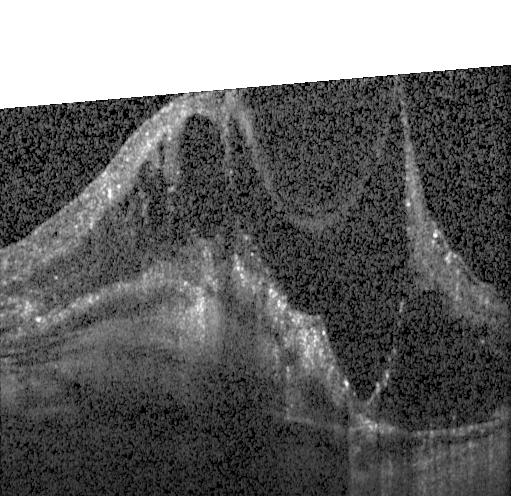

Diagnosis: a choroidal neovascular membrane.